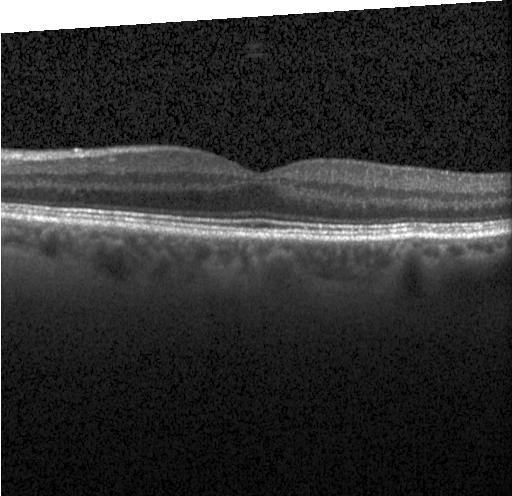

Acquired on a Heidelberg Spectralis; OCT B-scan — Impression: no choroidal neovascularization, no diabetic macular edema, and no drusen.